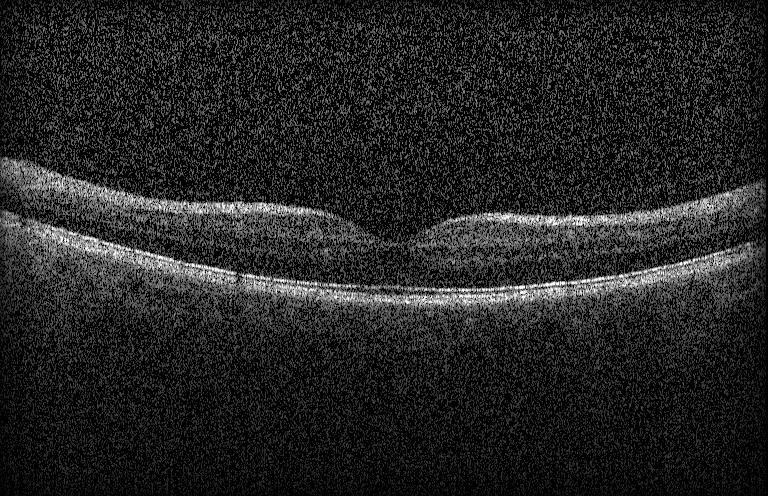
Retinal OCT cross-section showing no choroidal neovascularization, diabetic macular edema, or drusen.